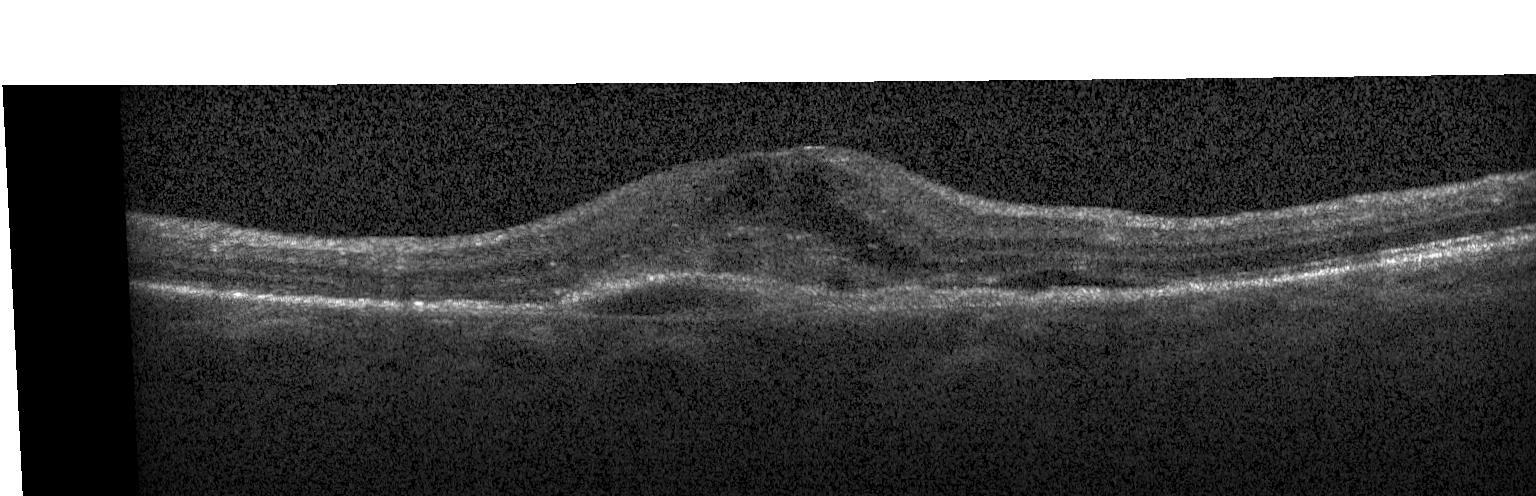 OCT line scan
This B-scan demonstrates a choroidal neovascular membrane.